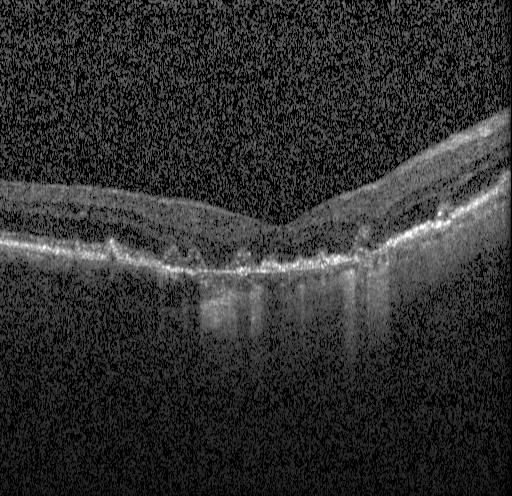 OCT B-scan showing choroidal neovascularization.